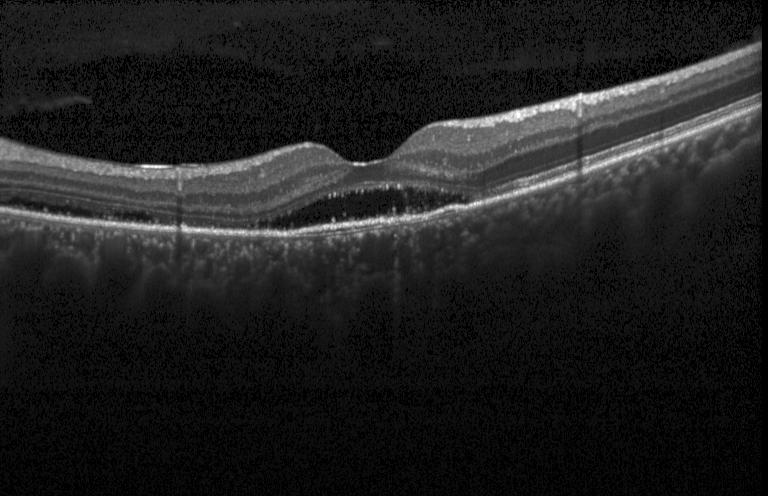 Macular scan. Retinal OCT B-scan
The scan shows choroidal neovascularization.